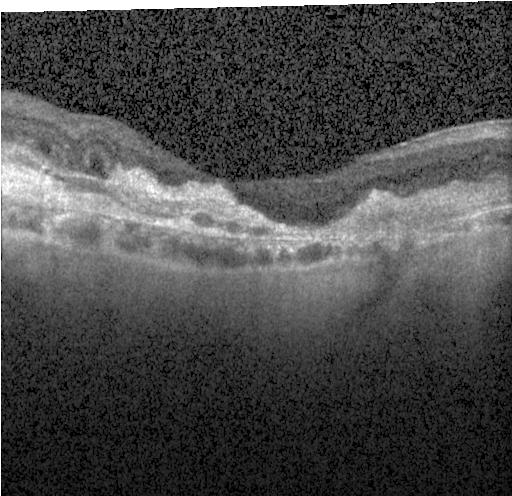
OCT B-scan showing a choroidal neovascular membrane.